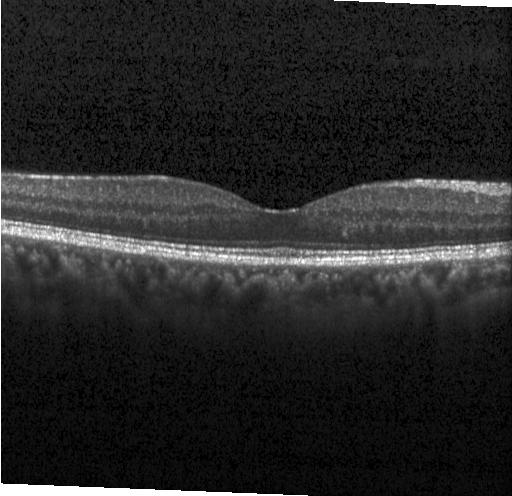 Finding: no choroidal neovascularization, no diabetic macular edema, and no drusen.